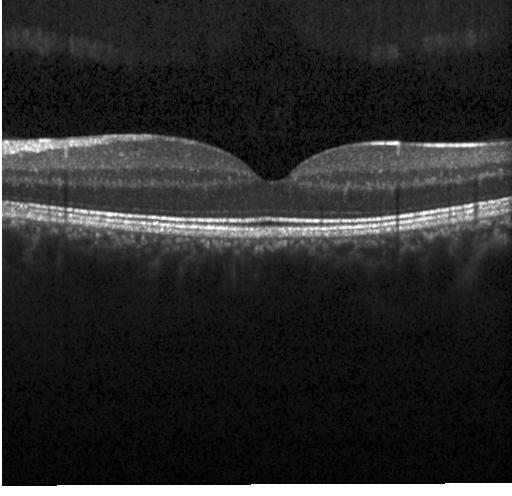

Assessment: no evidence of choroidal neovascularization, diabetic macular edema, or drusen.